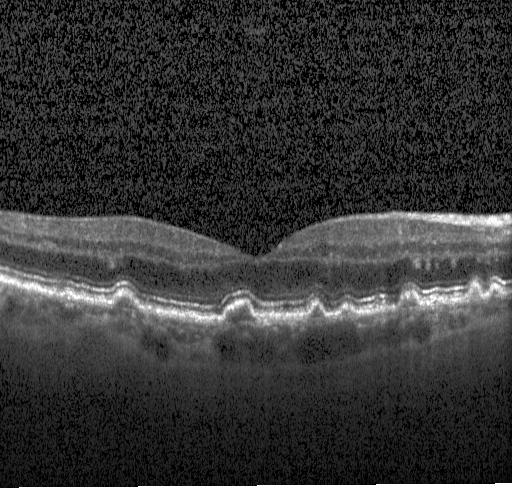

Horizontal scan through the fovea · SD-OCT · Heidelberg Spectralis · OCT line scan.
Impression: multiple drusen.